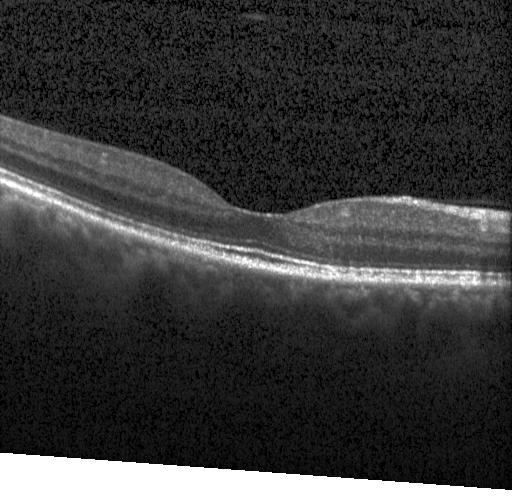 Dx: no evidence of choroidal neovascularization, diabetic macular edema, or drusen.